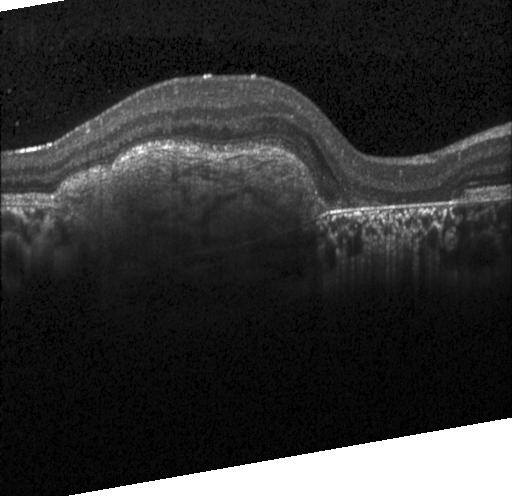

Impression: choroidal neovascularization (CNV).